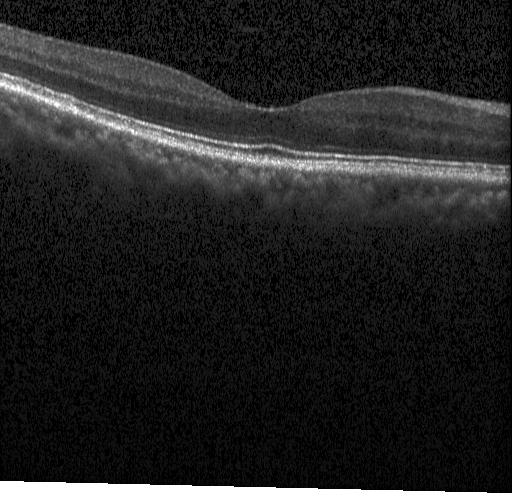 Spectral-domain OCT B-scan: neither CNV, DME, nor drusen.